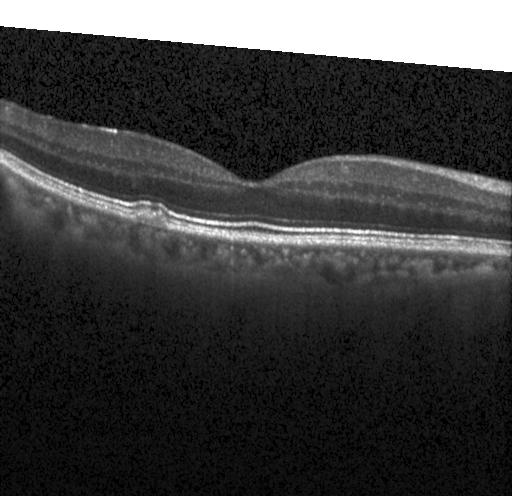 Retinal OCT B-scan, fovea-centered, SD-OCT, acquired on a Heidelberg Spectralis
This B-scan demonstrates multiple drusen.